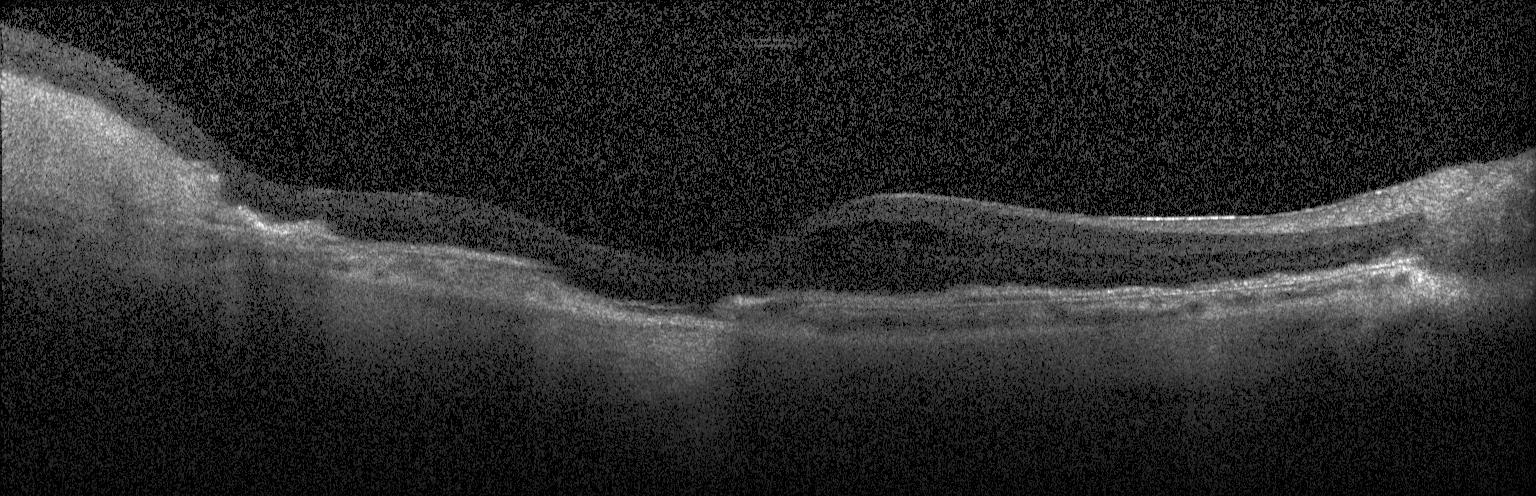 Optical coherence tomography scan.
The scan shows a choroidal neovascular membrane.